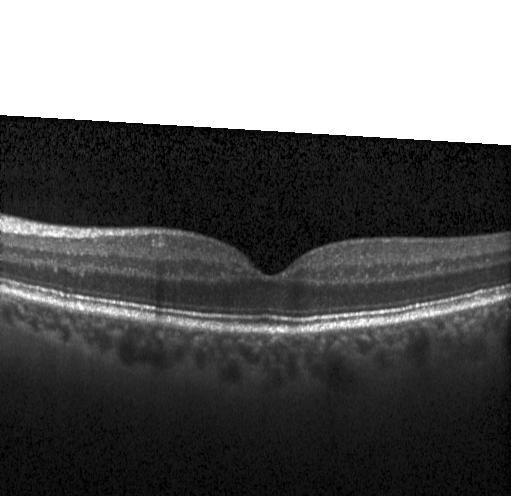 Spectral-domain optical coherence tomography, retinal OCT cross-section, horizontal scan through the fovea. Impression: no choroidal neovascularization, diabetic macular edema, or drusen.